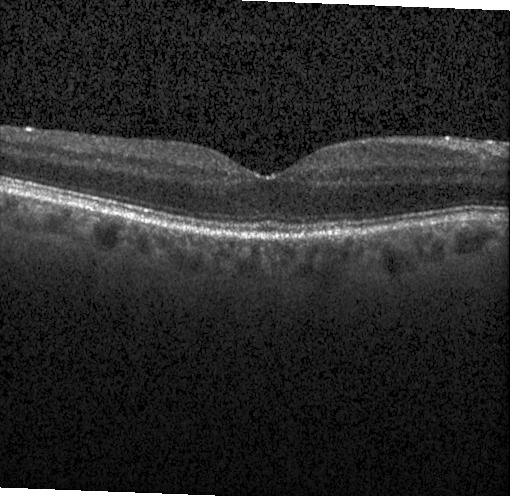
OCT B-scan showing no evidence of choroidal neovascularization, diabetic macular edema, or drusen.